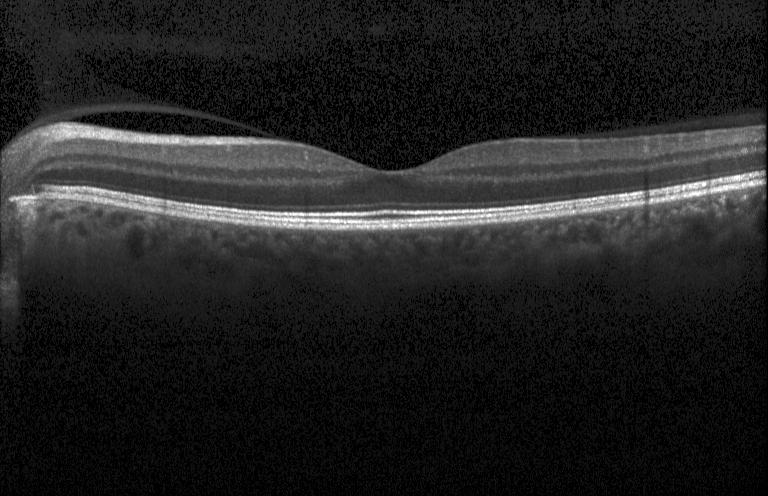 OCT B-scan showing neither choroidal neovascularization, diabetic macular edema, nor drusen.